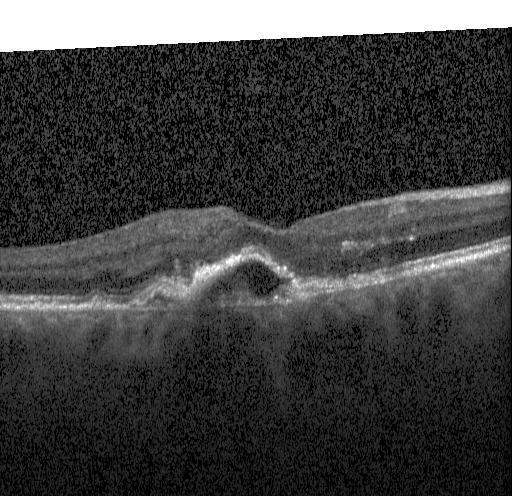 Dx: CNV.